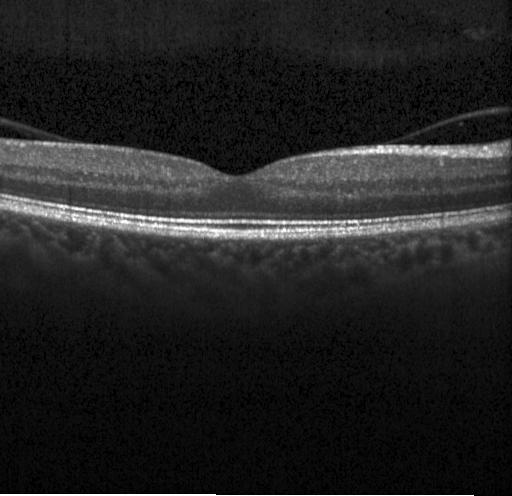 Finding: no choroidal neovascularization, no diabetic macular edema, and no drusen.